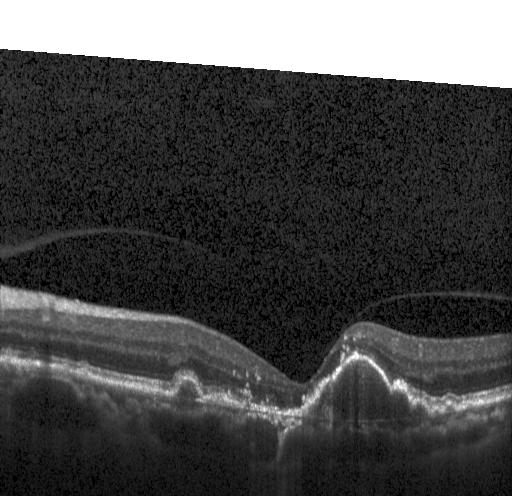

OCT B-scan · centered on the fovea.
Impression: a choroidal neovascular membrane.